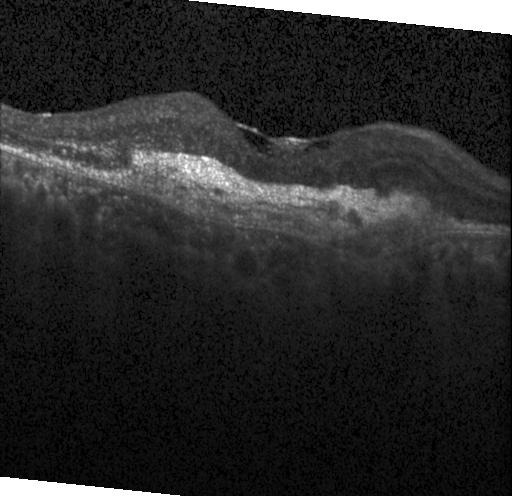 Heidelberg Spectralis OCT system, macular scan, OCT line scan, SD-OCT
Assessment: a choroidal neovascular membrane.